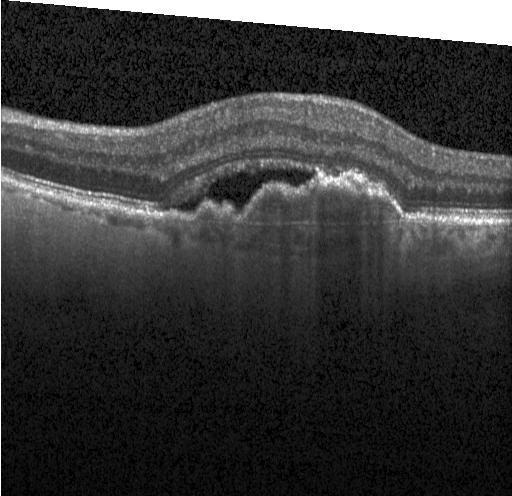
Dx: a choroidal neovascular membrane.